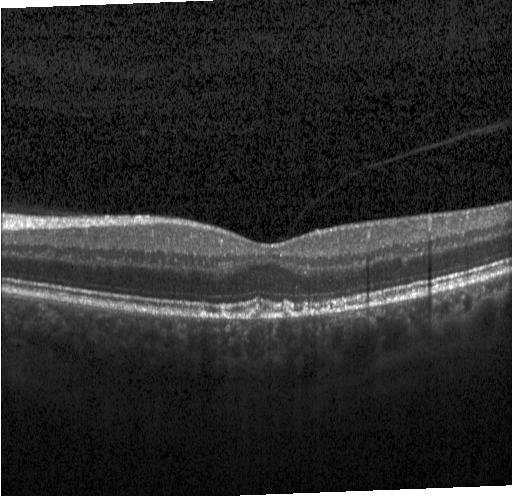
Optical coherence tomography B-scan · spectral-domain optical coherence tomography — Sub-RPE drusenoid deposits.